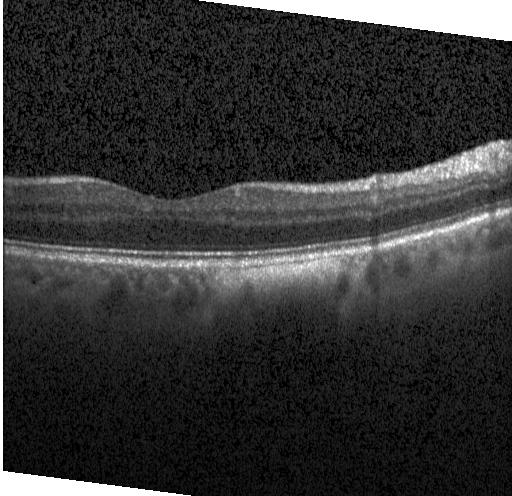 OCT finding: neither CNV, DME, nor drusen.